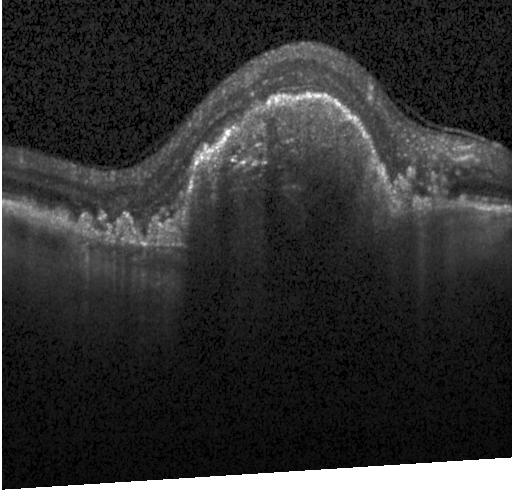

Retinal OCT B-scan, macular scan, instrument: Heidelberg Spectralis. This B-scan demonstrates choroidal neovascularization.